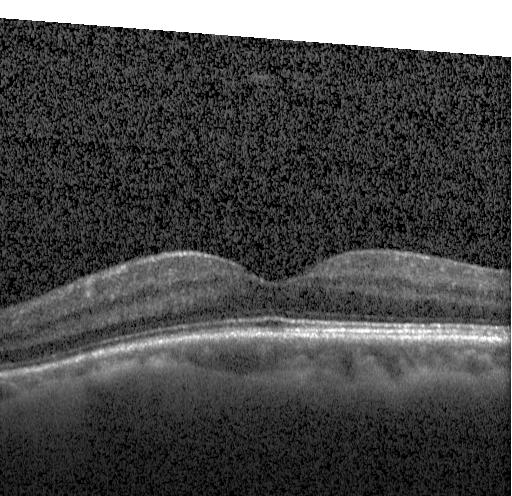 Instrument: Heidelberg Spectralis; horizontal scan through the fovea; retinal OCT cross-section.
Impression: no evidence of choroidal neovascularization, diabetic macular edema, or drusen.